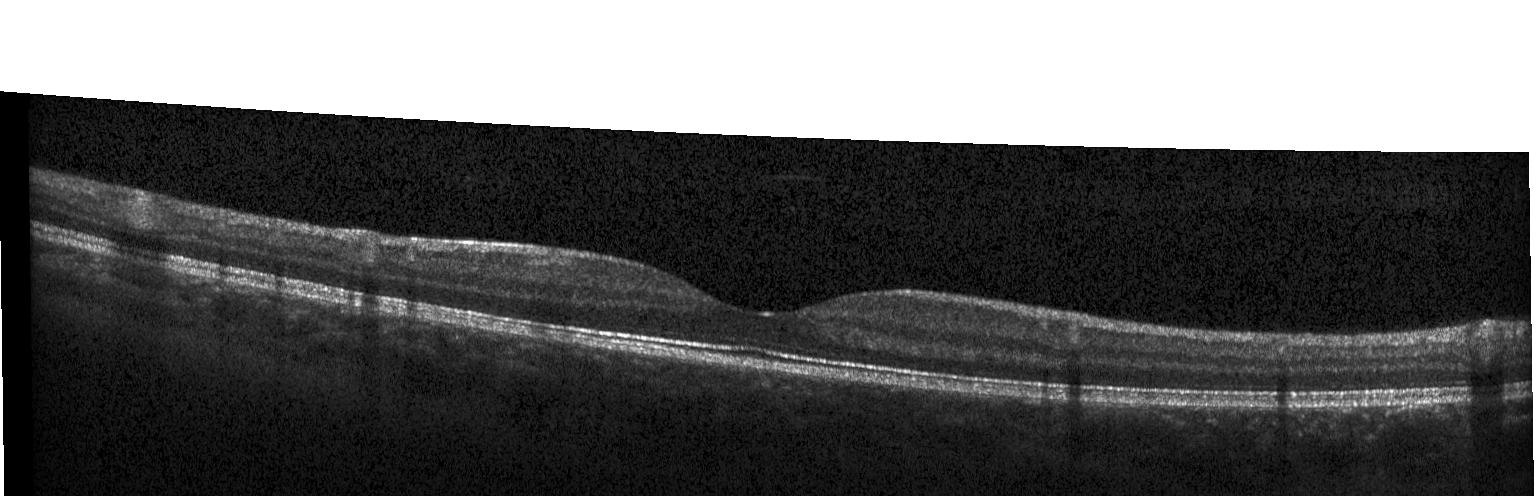
SD-OCT; acquired on a Heidelberg Spectralis; fovea-centered; OCT line scan
OCT finding: no evidence of choroidal neovascularization, diabetic macular edema, or drusen.